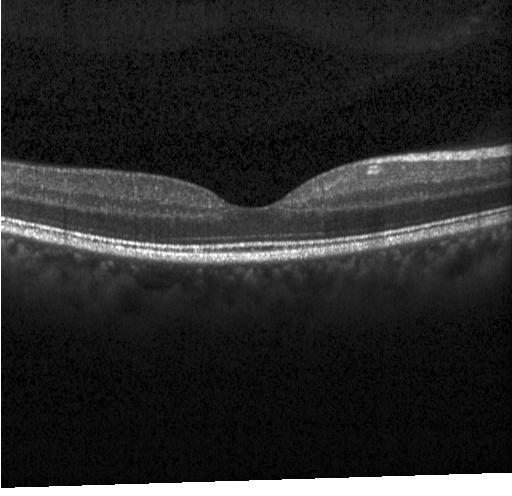 Impression: neither choroidal neovascularization, diabetic macular edema, nor drusen.